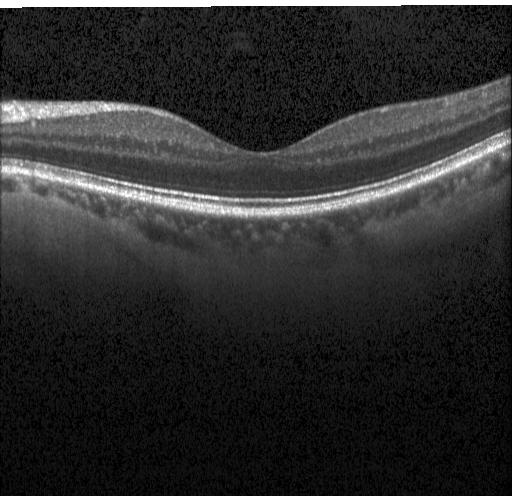 Spectral-domain OCT · acquired on a Heidelberg Spectralis · retinal OCT cross-section · fovea-centered
No CNV, DME, or drusen.